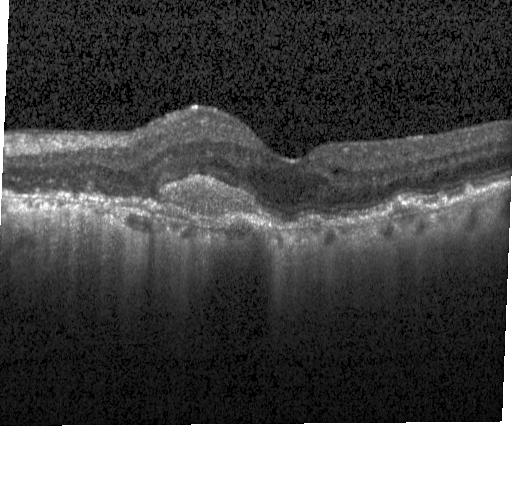 Macular scan, retinal OCT B-scan — Impression: a choroidal neovascular membrane.